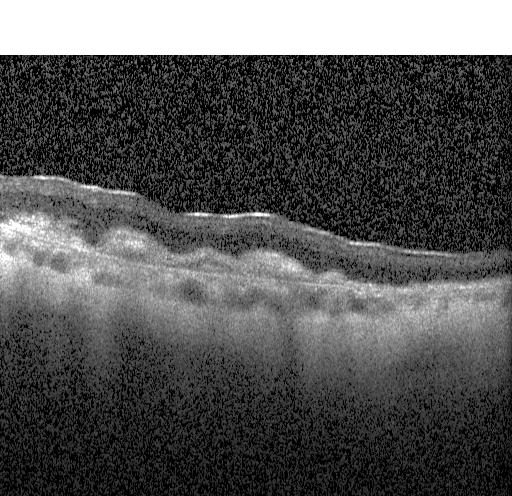 Dx: choroidal neovascularization.